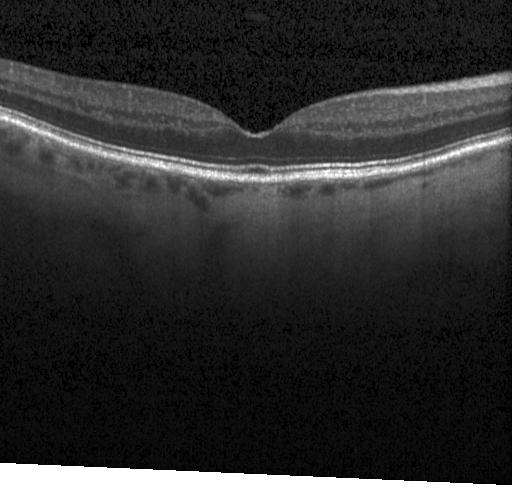
Macular OCT demonstrating neither CNV, DME, nor drusen.